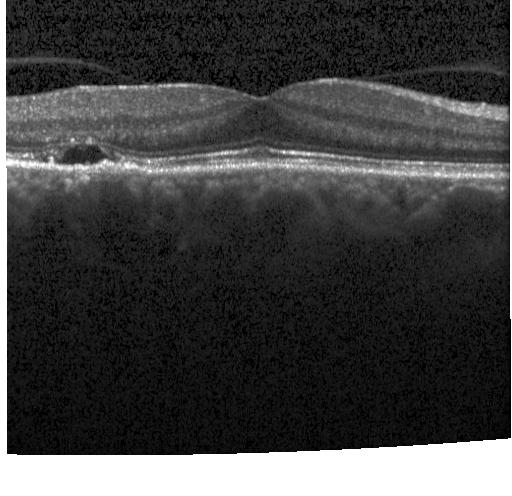 Finding: a choroidal neovascular membrane.